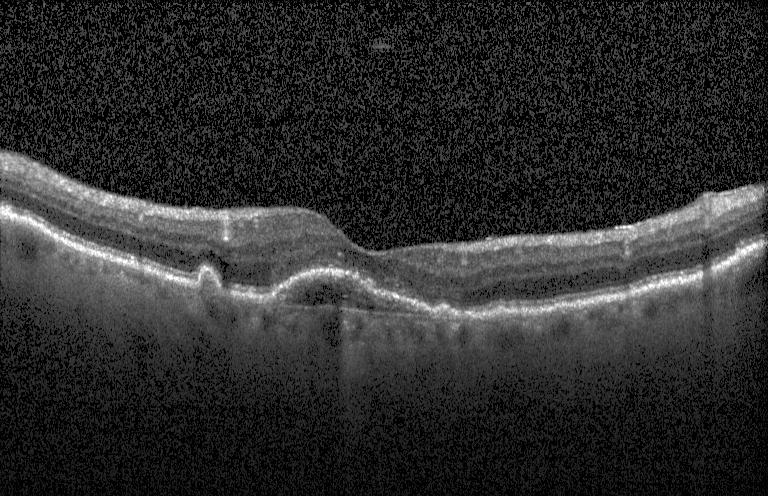
Finding: CNV.